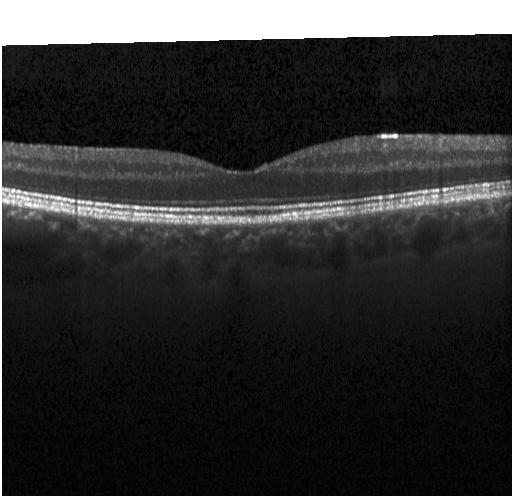
SD-OCT, fovea-centered, optical coherence tomography scan. Impression: no choroidal neovascularization, diabetic macular edema, or drusen.